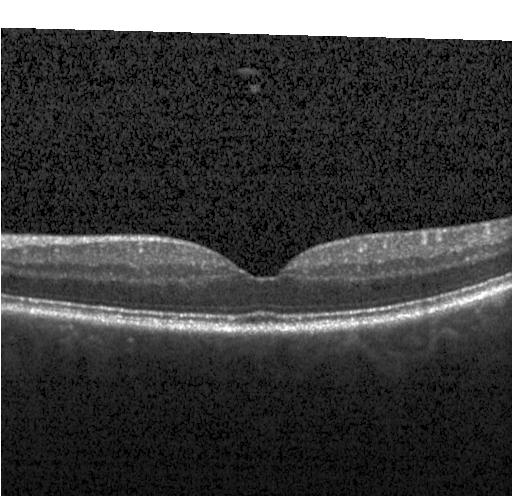
Impression: neither CNV, DME, nor drusen.